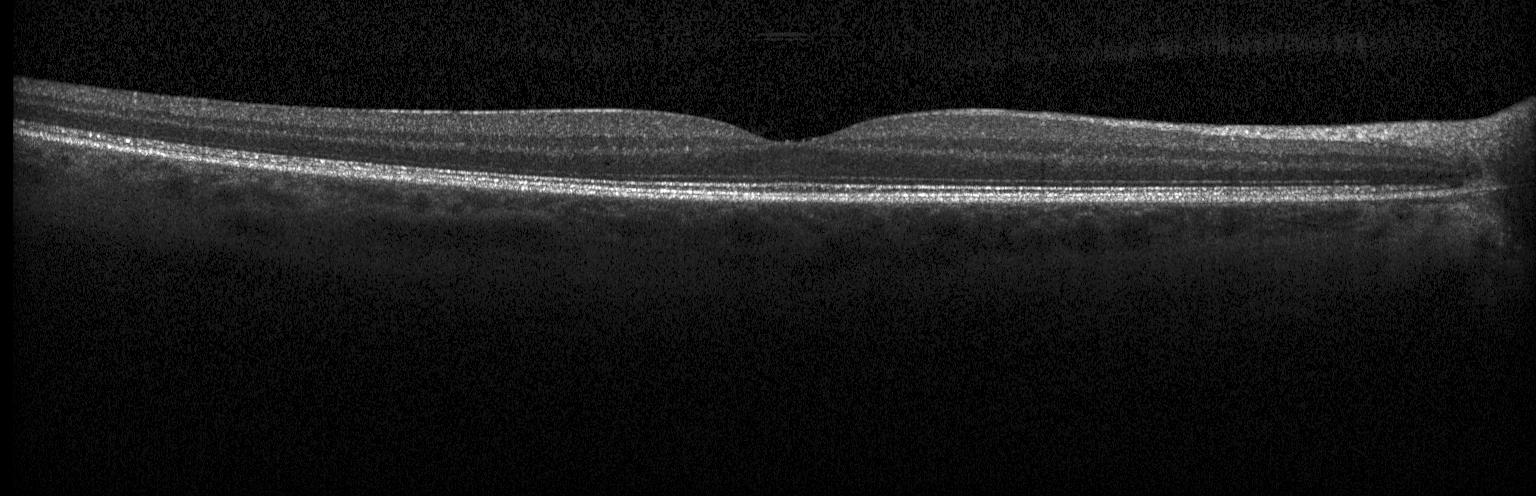
Finding: neither choroidal neovascularization, diabetic macular edema, nor drusen.